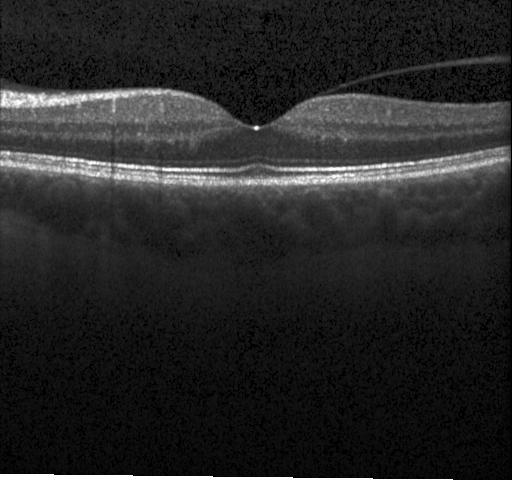 OCT scan showing neither choroidal neovascularization, diabetic macular edema, nor drusen.